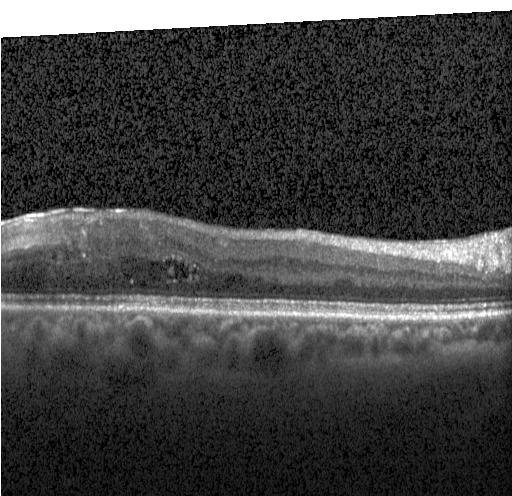

The scan shows DME.